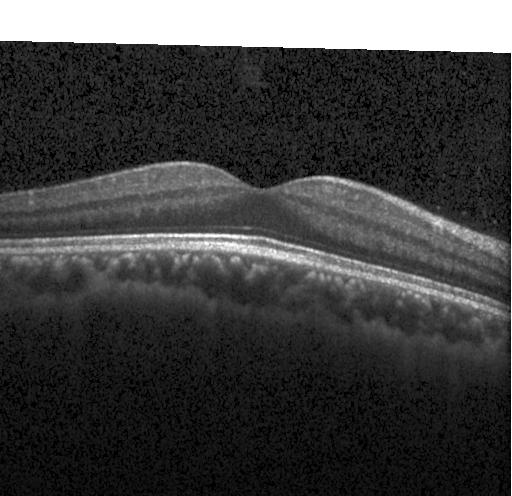 Optical coherence tomography scan. Macular OCT: no evidence of choroidal neovascularization, diabetic macular edema, or drusen.